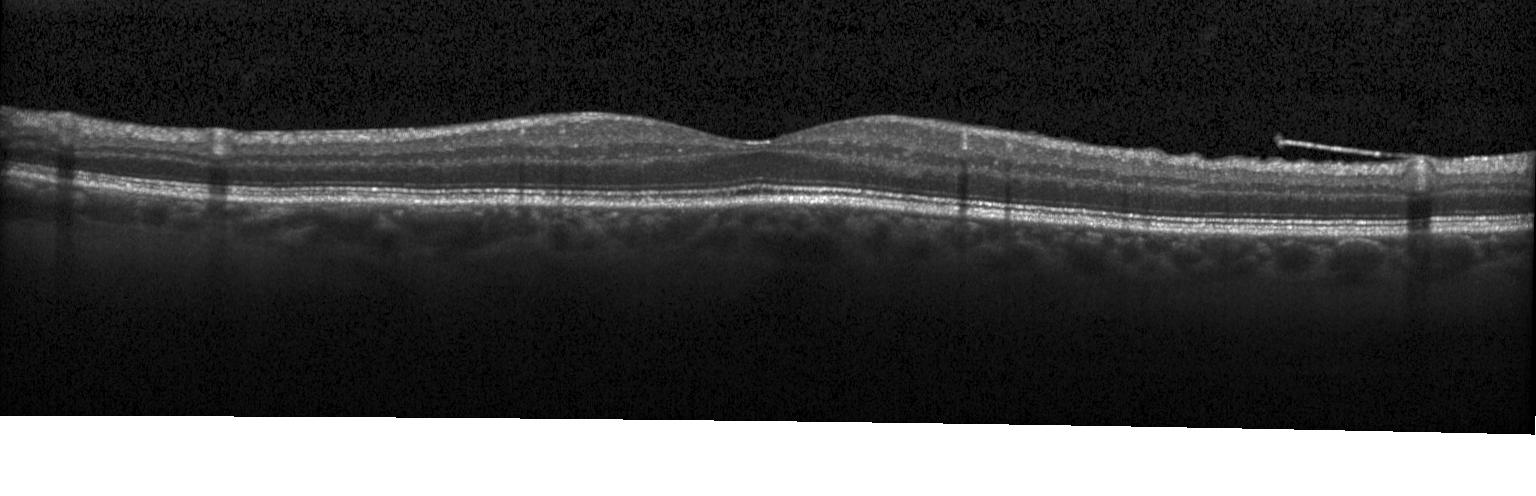
Spectral-domain OCT. Retinal OCT B-scan — Impression: no choroidal neovascularization, diabetic macular edema, or drusen.